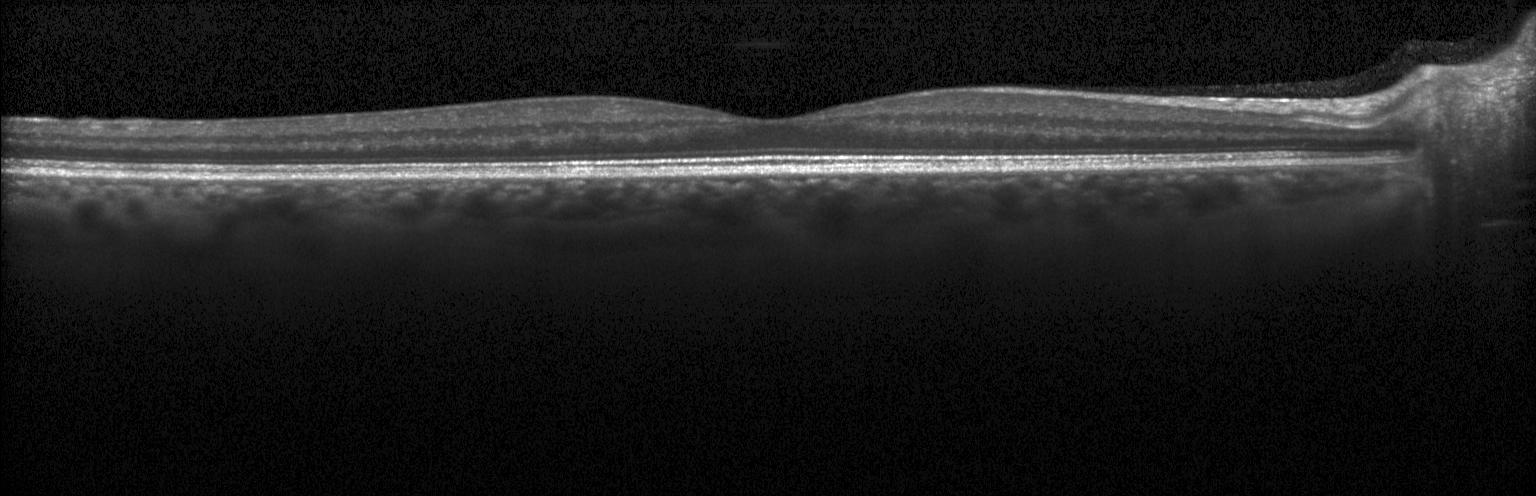 Macular OCT demonstrating no CNV, DME, or drusen.